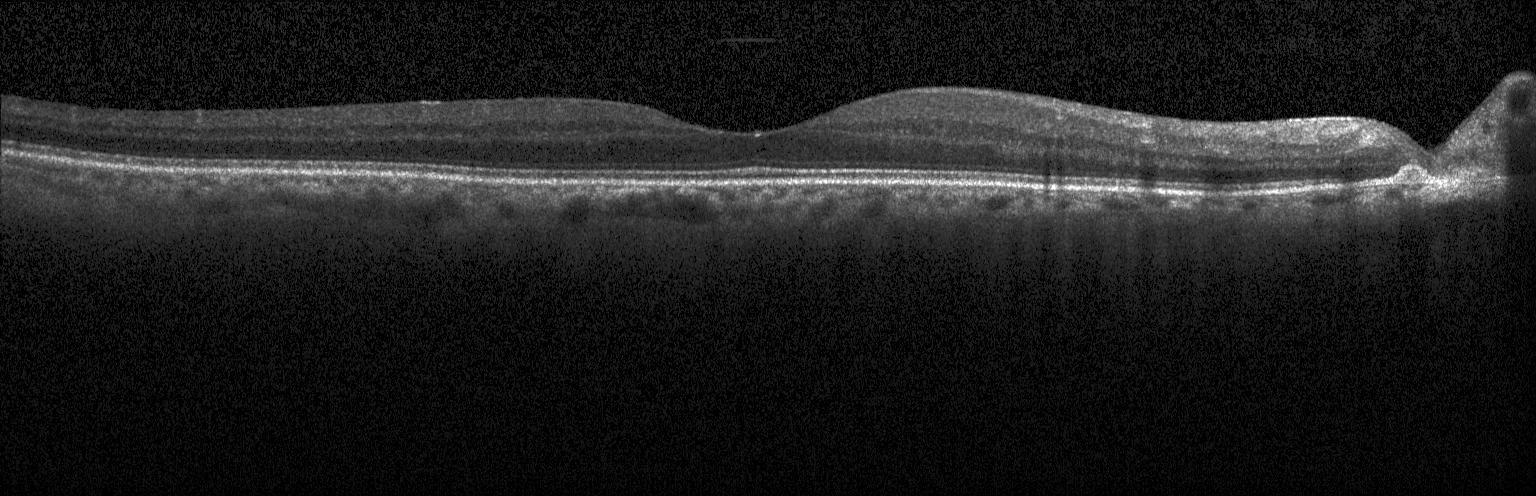

Retinal OCT cross-section — Neither choroidal neovascularization, diabetic macular edema, nor drusen.